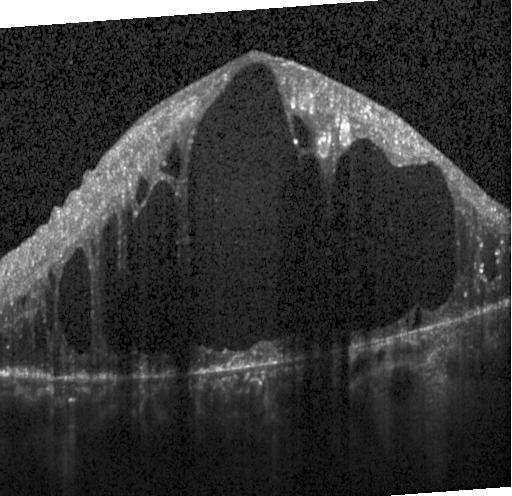

Assessment: diabetic macular edema (DME).